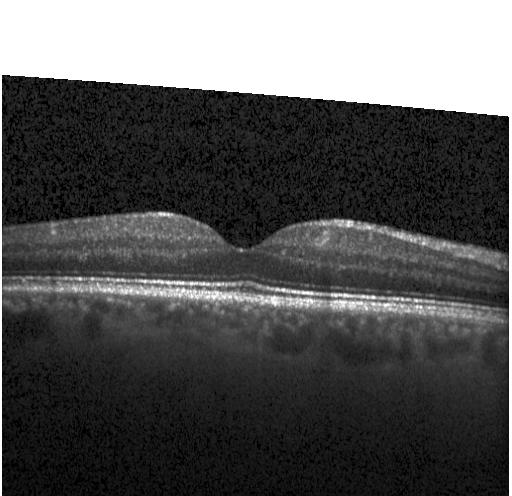
Impression: no evidence of choroidal neovascularization, diabetic macular edema, or drusen.